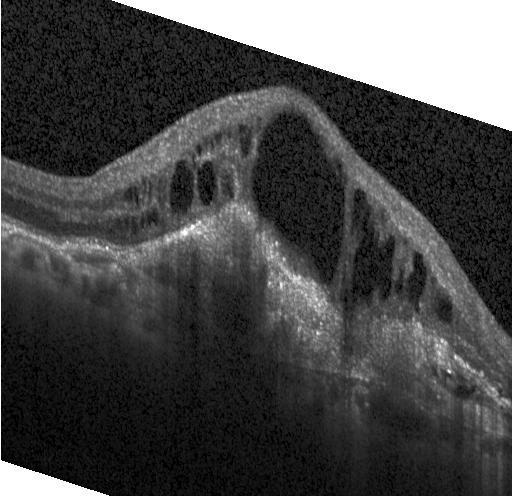

Optical coherence tomography scan, acquired on a Heidelberg Spectralis, macular scan, spectral-domain optical coherence tomography
This B-scan demonstrates a choroidal neovascular membrane.